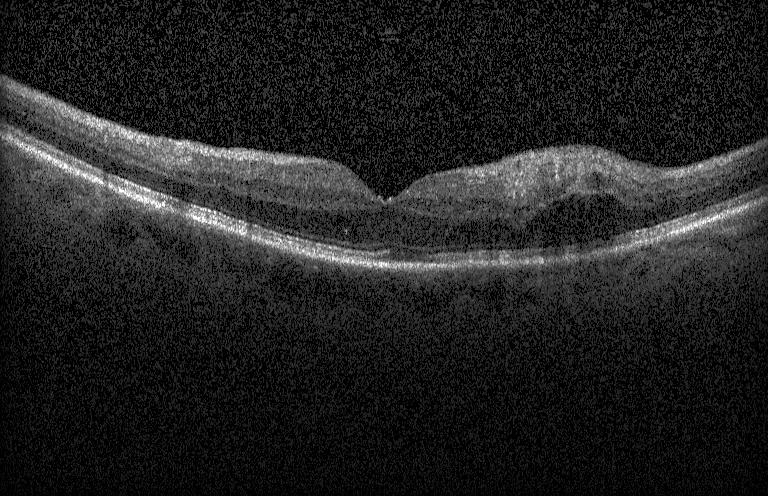
Spectral-domain OCT B-scan: diabetic macular edema (DME).